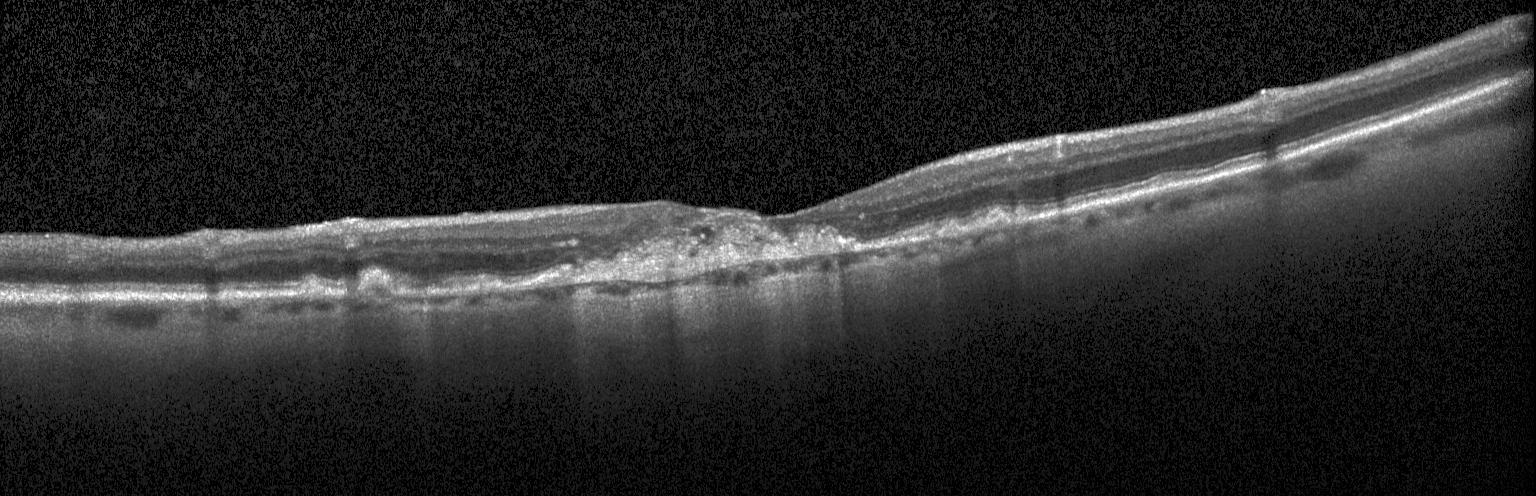
Macular OCT: choroidal neovascularization (CNV).